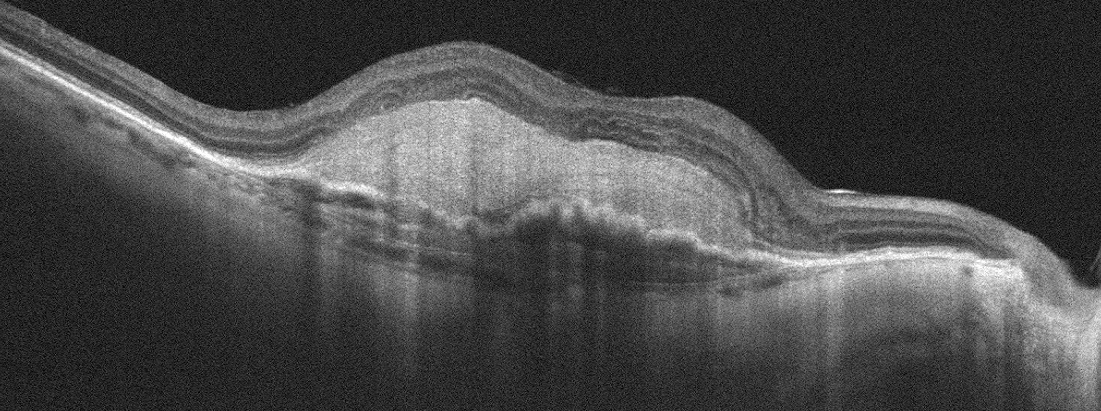

OCT finding: AMD.